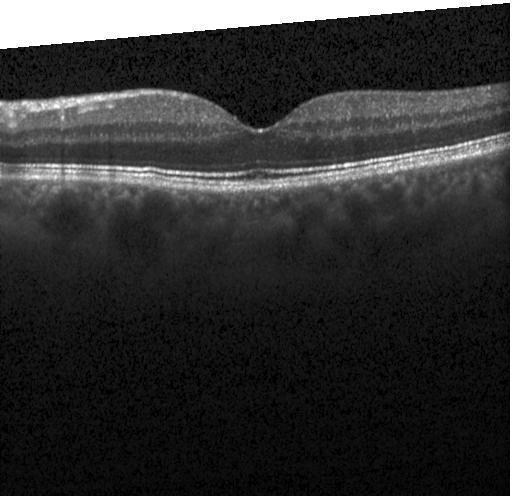

No evidence of choroidal neovascularization, diabetic macular edema, or drusen.